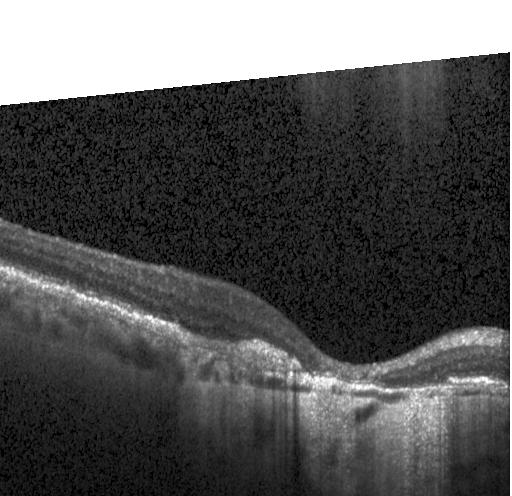
Diagnosis: choroidal neovascularization.